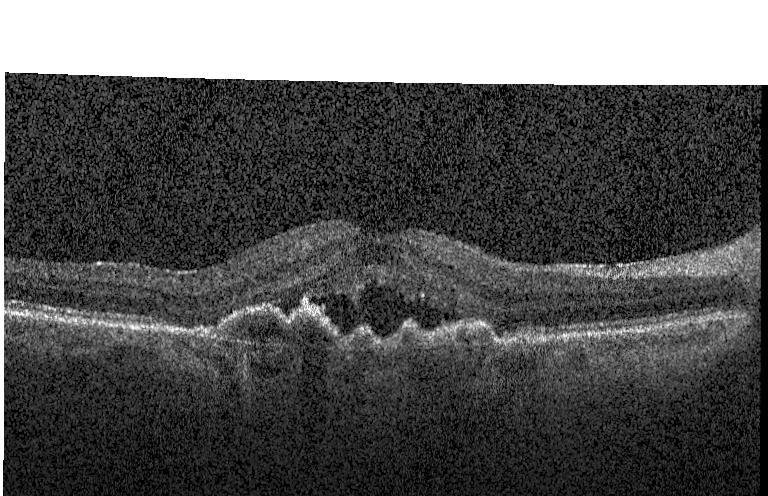
Spectral-domain OCT B-scan: a choroidal neovascular membrane.